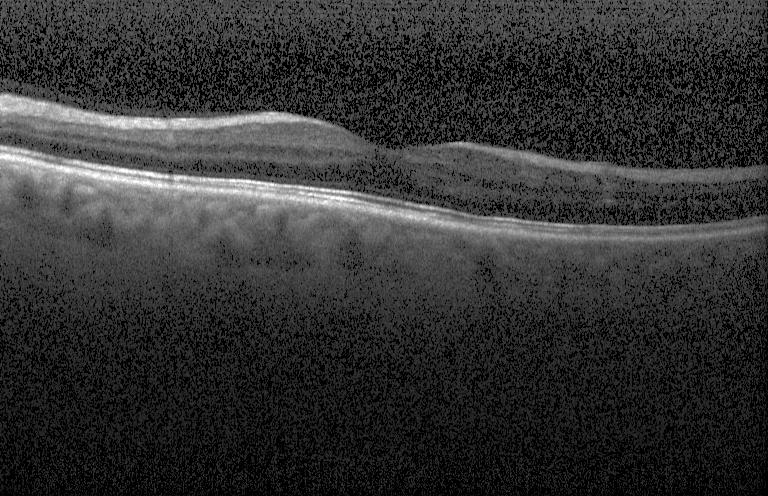
Macular OCT: neither choroidal neovascularization, diabetic macular edema, nor drusen.